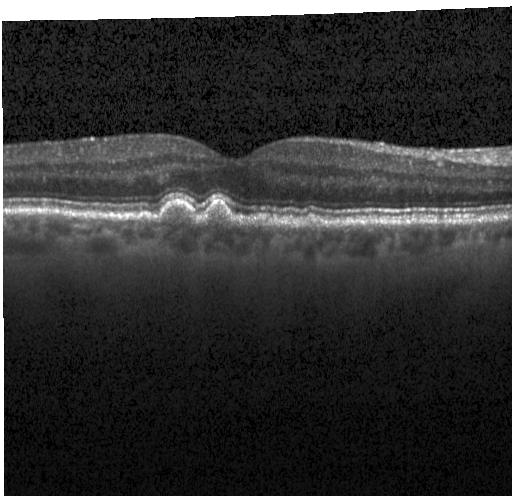
OCT scan showing multiple drusen.